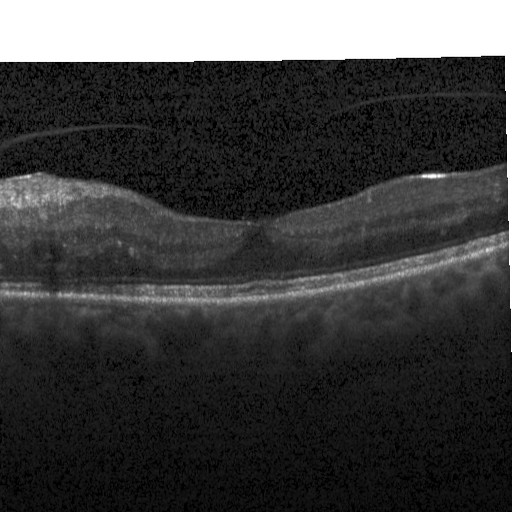
Heidelberg Spectralis OCT system. OCT B-scan. Horizontal scan through the fovea
Dx: DME.